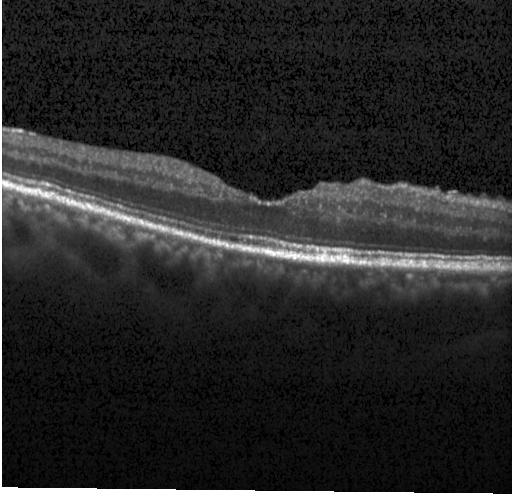

OCT scan showing no choroidal neovascularization, no diabetic macular edema, and no drusen.